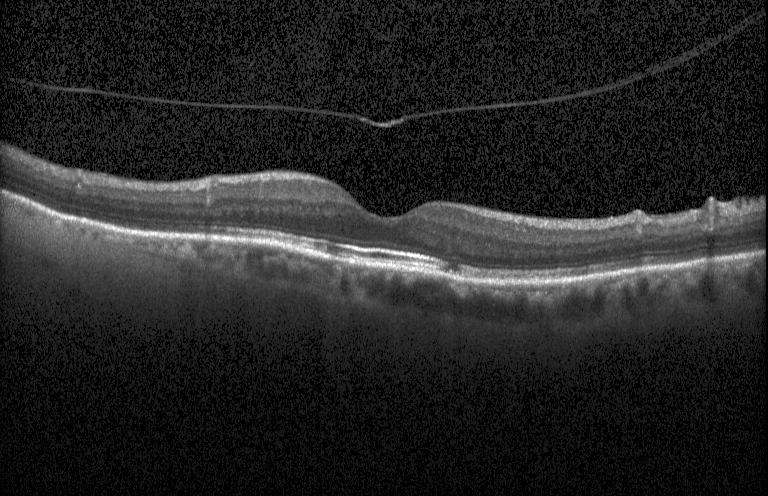

Retinal OCT B-scan.
Dx: neither CNV, DME, nor drusen.